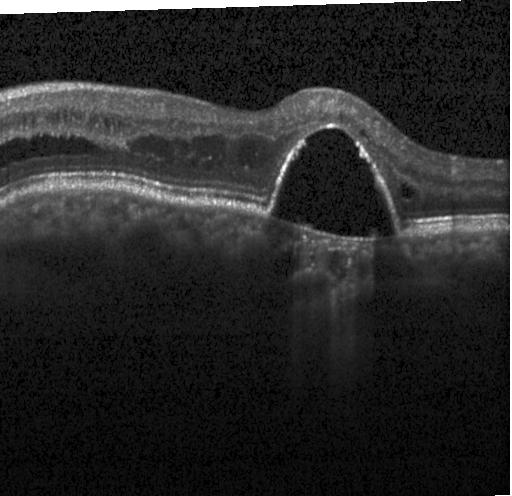

Retinal OCT cross-section, Heidelberg Spectralis. Diagnosis: CNV.